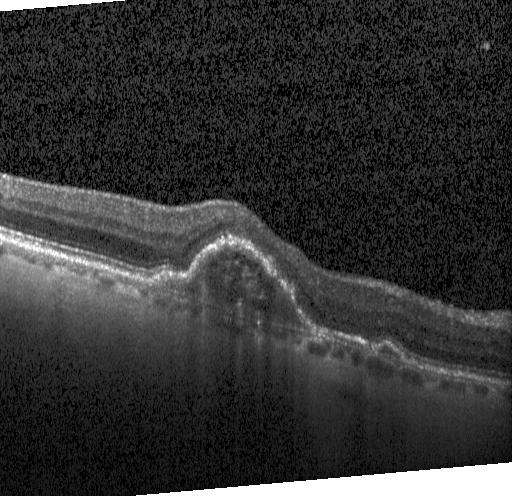
Macular OCT demonstrating a choroidal neovascular membrane.